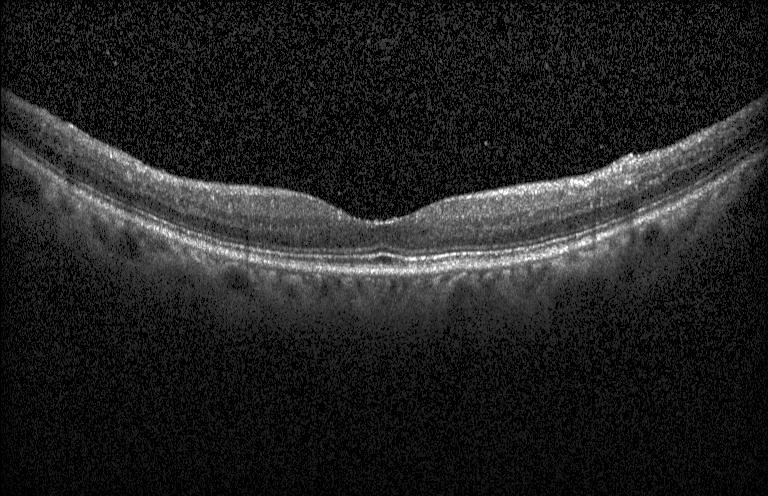 Optical coherence tomography scan. Instrument: Heidelberg Spectralis.
Assessment: no evidence of choroidal neovascularization, diabetic macular edema, or drusen.